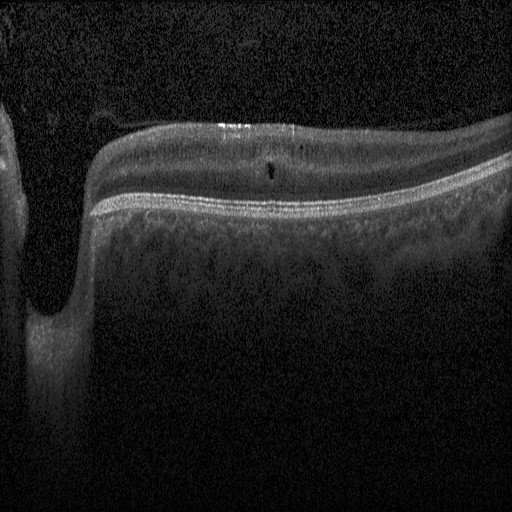

Fovea-centered, instrument: Heidelberg Spectralis, retinal OCT B-scan, spectral-domain OCT
The scan shows diabetic macular edema (DME).